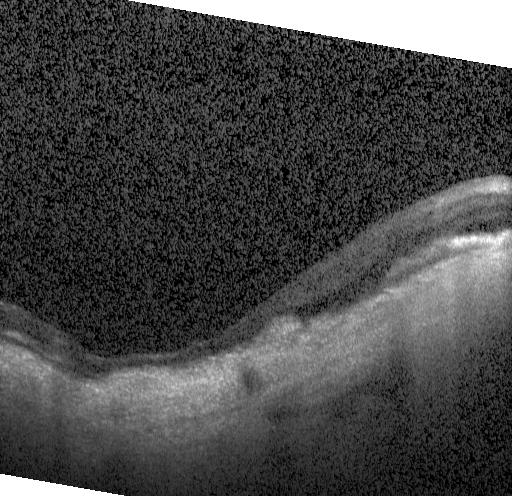
Fovea-centered. OCT B-scan. SD-OCT. Instrument: Heidelberg Spectralis
Dx: choroidal neovascularization.